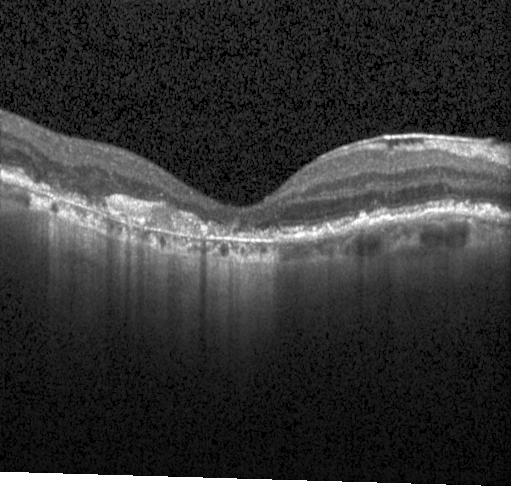
Horizontal scan through the fovea · retinal OCT B-scan · instrument: Heidelberg Spectralis. Choroidal neovascularization.